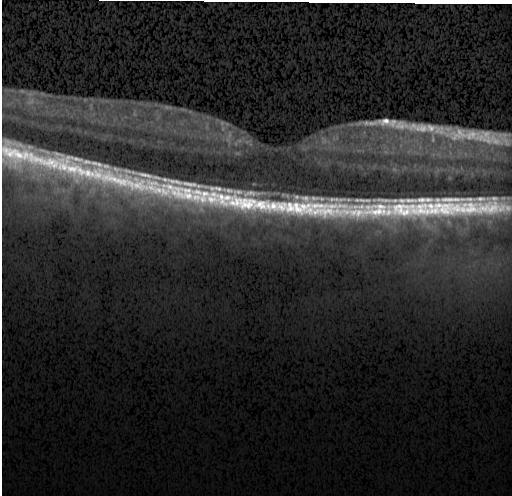 Dx: no choroidal neovascularization, no diabetic macular edema, and no drusen.